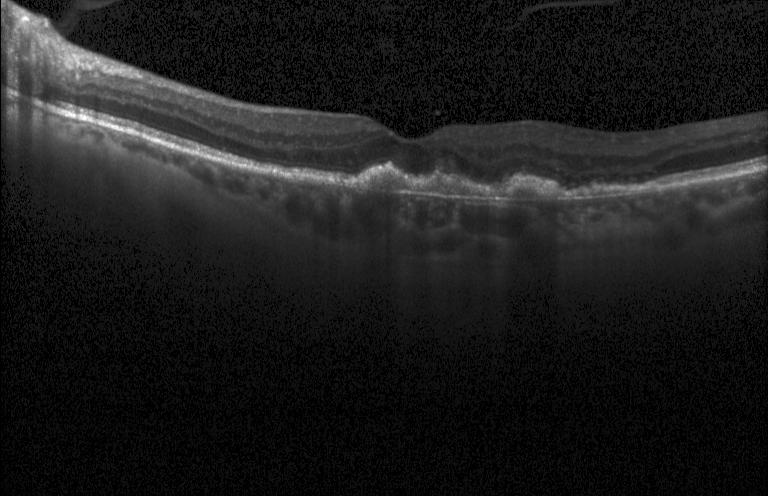

OCT scan showing choroidal neovascularization.